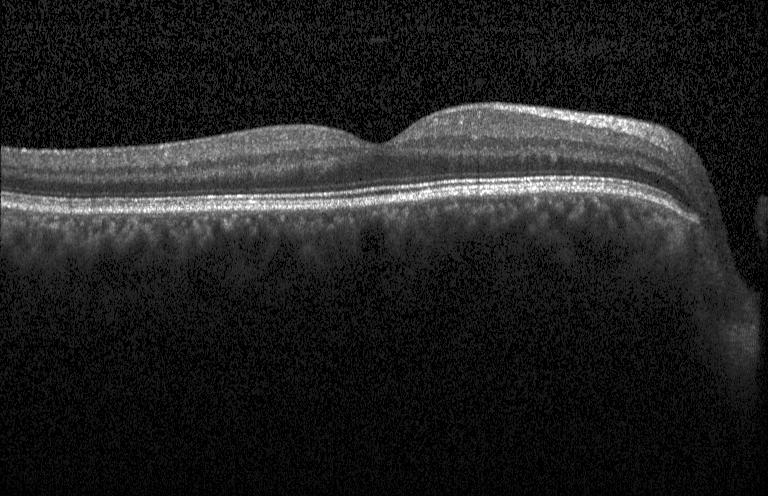
Horizontal scan through the fovea · OCT B-scan — Assessment: no evidence of CNV, DME, or drusen.